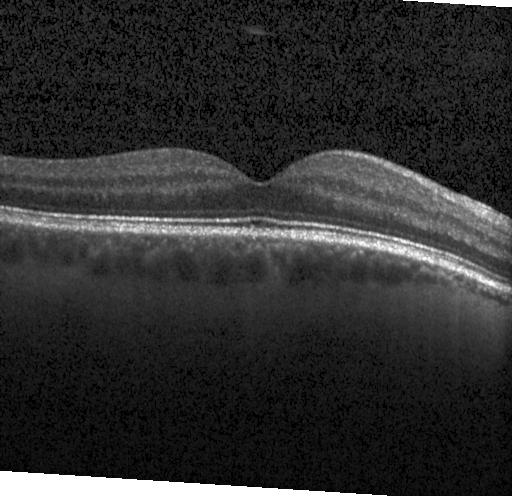

OCT B-scan.
Finding: no CNV, DME, or drusen.